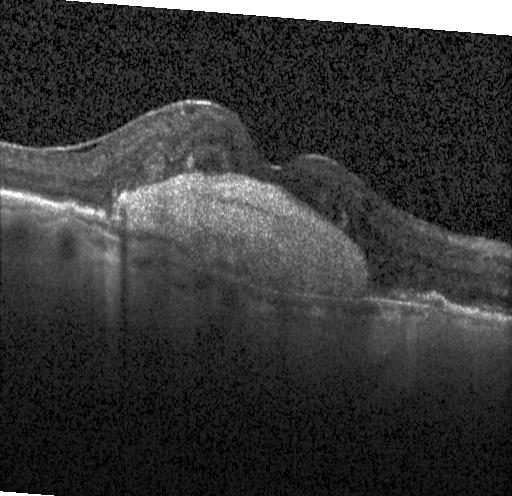
Heidelberg Spectralis. Macular scan. Optical coherence tomography B-scan. Impression: choroidal neovascularization (CNV).